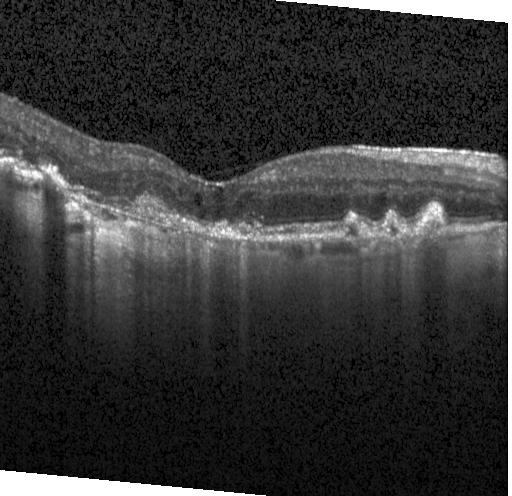

Finding: choroidal neovascularization.